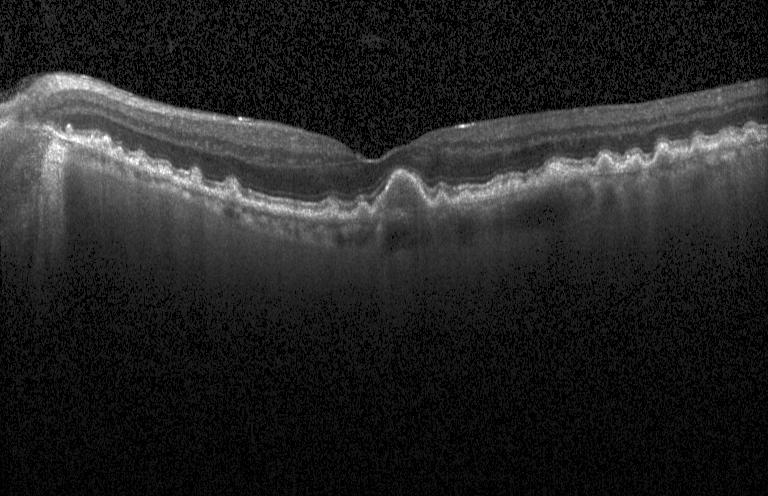
Retinal OCT cross-section. Assessment: drusen.